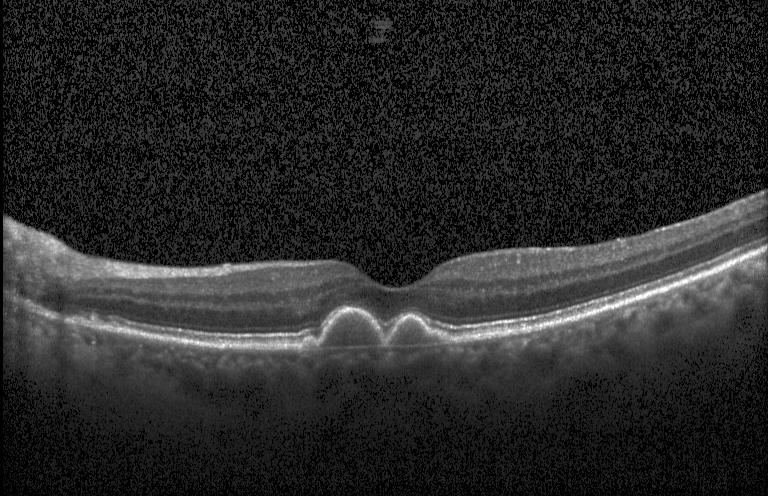 OCT B-scan showing drusen.